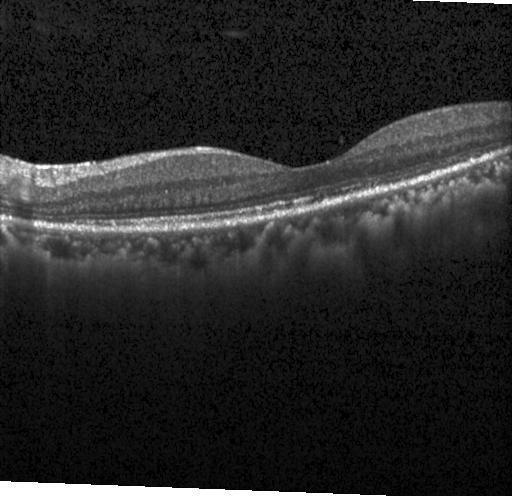
Macular scan; instrument: Heidelberg Spectralis; spectral-domain optical coherence tomography; OCT B-scan
Diagnosis: no choroidal neovascularization, no diabetic macular edema, and no drusen.